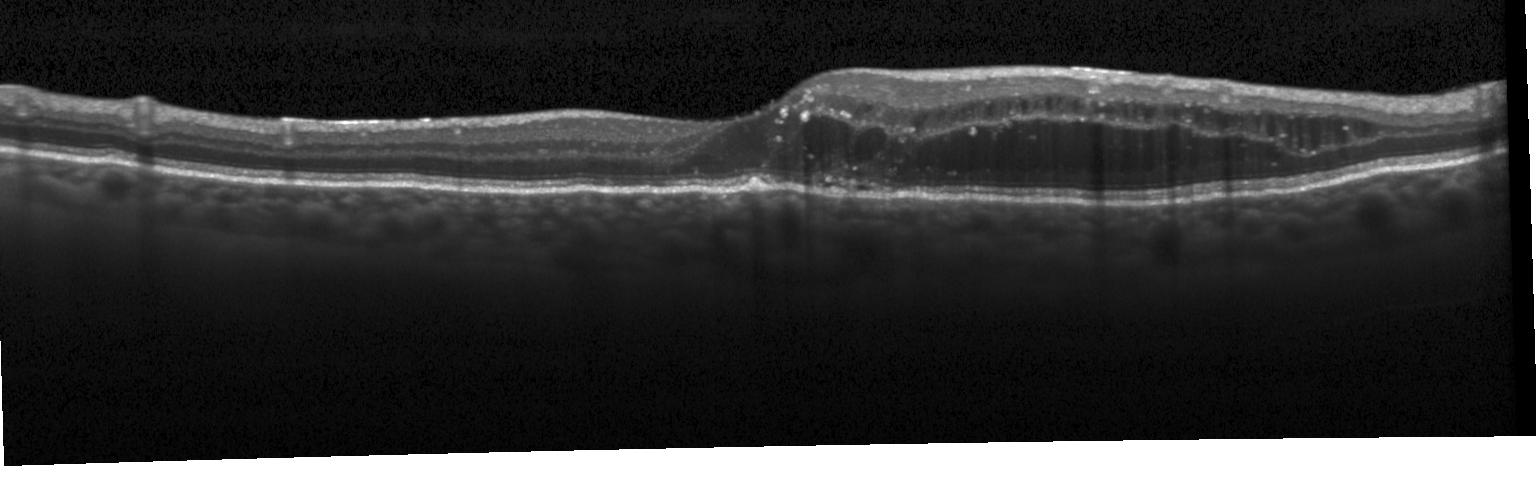

Fovea-centered · retinal OCT cross-section. Dx: diabetic macular edema.